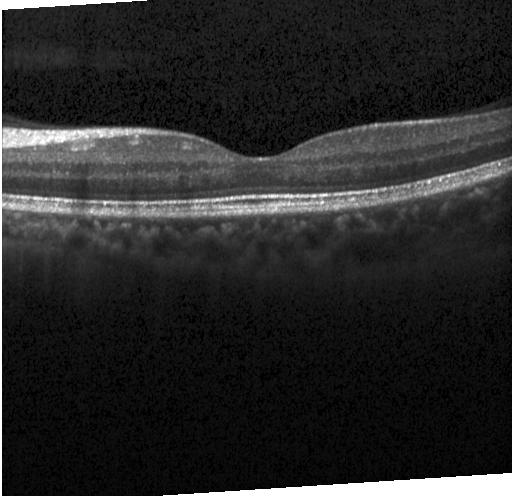 Instrument: Heidelberg Spectralis. OCT line scan. Macular scan. SD-OCT.
Finding: no evidence of choroidal neovascularization, diabetic macular edema, or drusen.